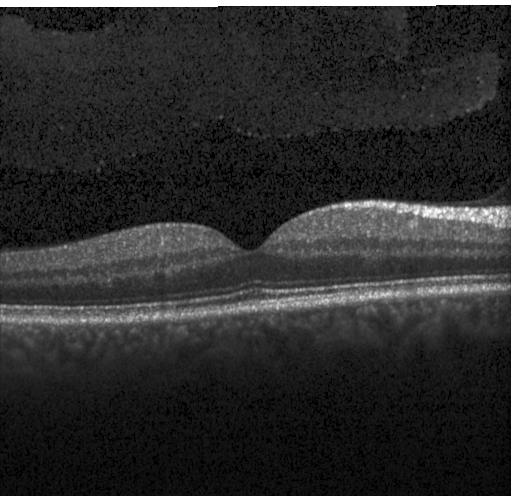
Optical coherence tomography B-scan — Impression: no evidence of choroidal neovascularization, diabetic macular edema, or drusen.